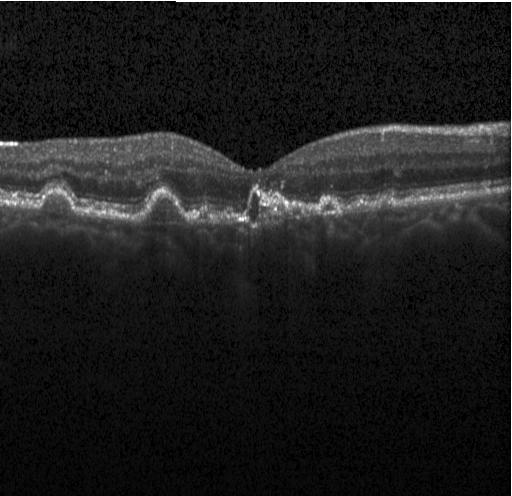
Impression: a choroidal neovascular membrane.